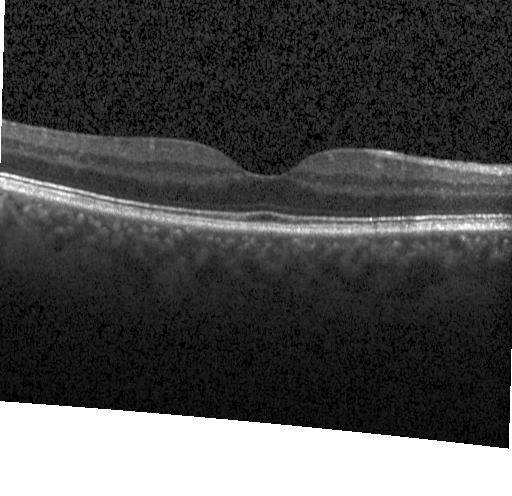 OCT line scan.
Finding: neither choroidal neovascularization, diabetic macular edema, nor drusen.